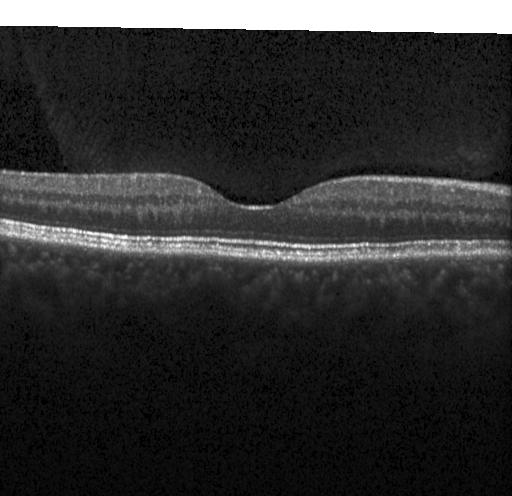 Centered on the fovea, OCT B-scan.
No evidence of choroidal neovascularization, diabetic macular edema, or drusen.